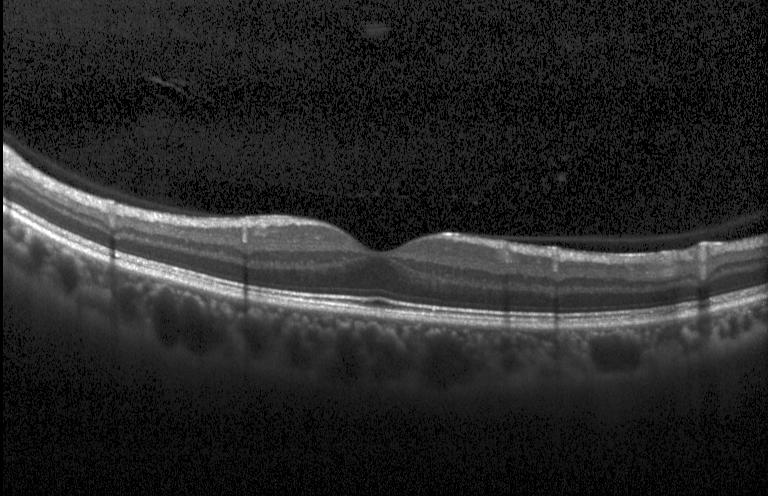

Diagnosis: no CNV, no DME, and no drusen.